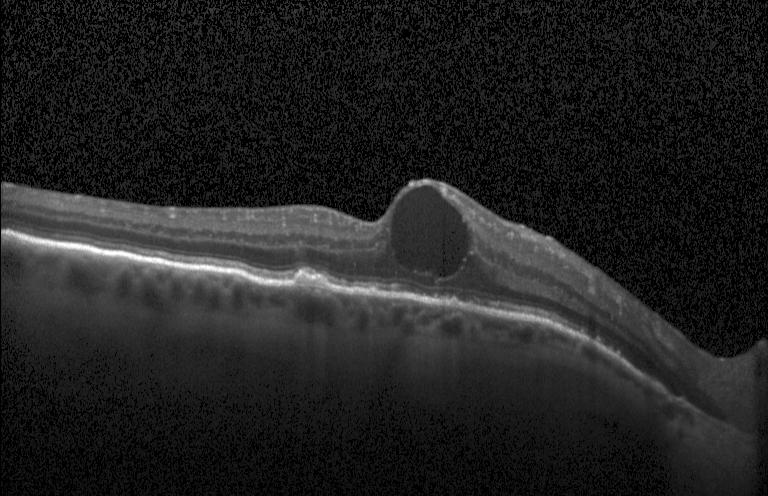

Retinal OCT B-scan.
Dx: a choroidal neovascular membrane.